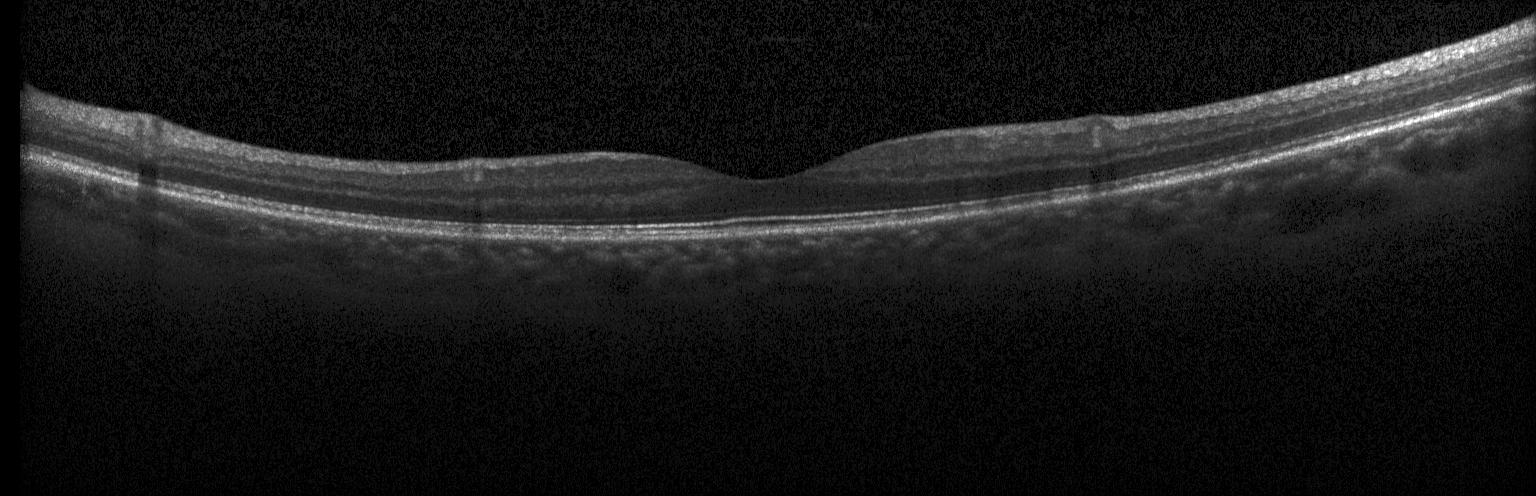

Optical coherence tomography B-scan. Assessment: no choroidal neovascularization, no diabetic macular edema, and no drusen.